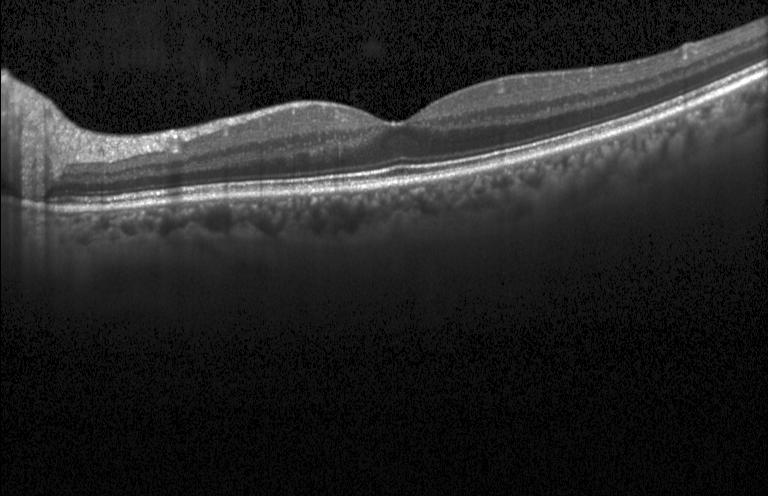
Diagnosis: neither choroidal neovascularization, diabetic macular edema, nor drusen.